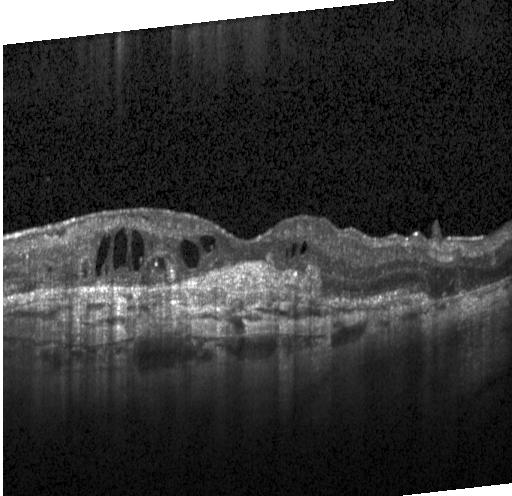

Acquired on a Heidelberg Spectralis; retinal OCT B-scan — Impression: a choroidal neovascular membrane.